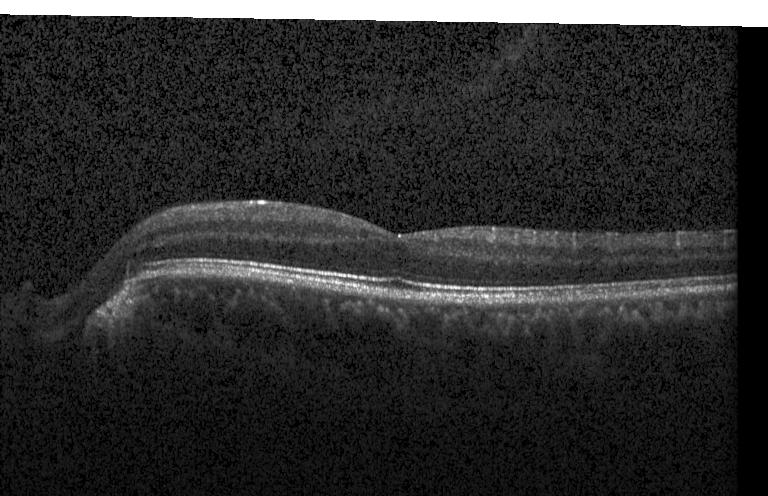 Retinal OCT B-scan. Heidelberg Spectralis OCT system. Impression: no choroidal neovascularization, diabetic macular edema, or drusen.